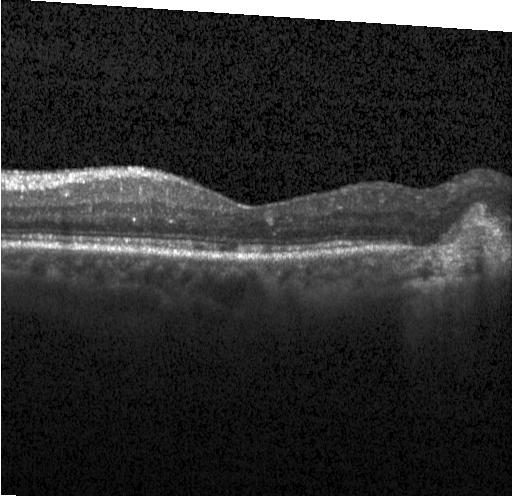

Optical coherence tomography B-scan. A choroidal neovascular membrane.